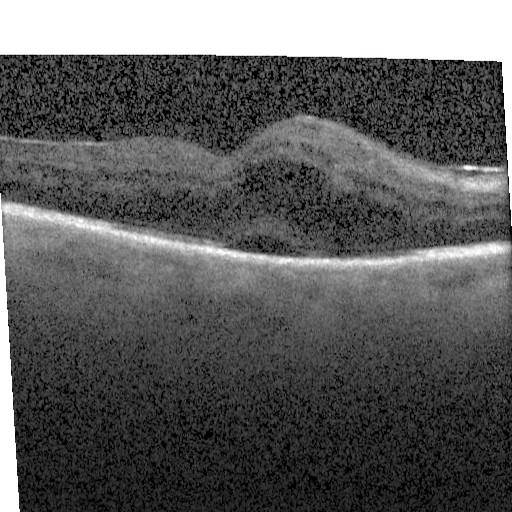

OCT finding: diabetic macular edema (DME).